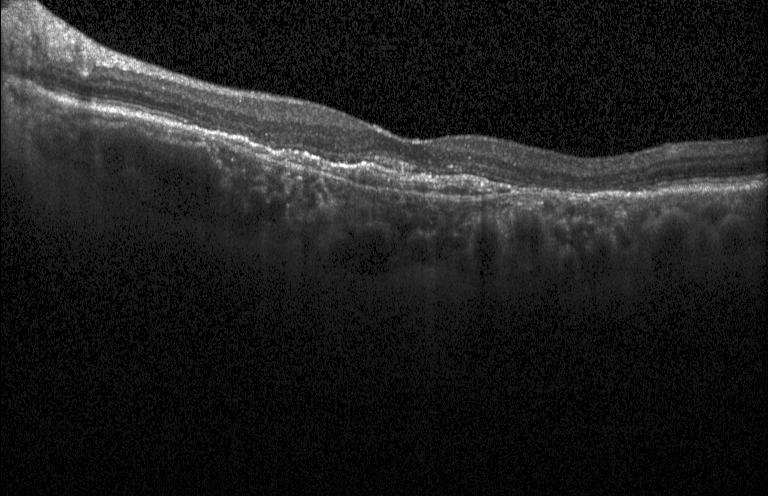
Diagnosis: a choroidal neovascular membrane.